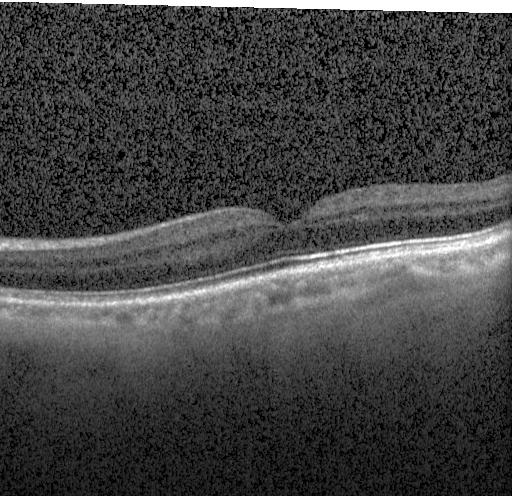 Spectral-domain OCT. Optical coherence tomography scan. Centered on the fovea. Heidelberg Spectralis OCT system.
Impression: no CNV, no DME, and no drusen.